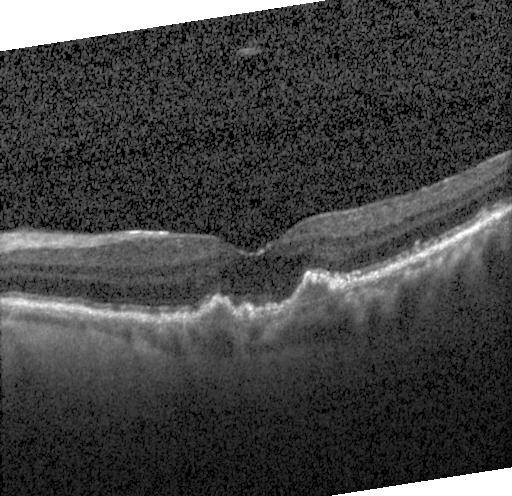 Diagnosis: a choroidal neovascular membrane.